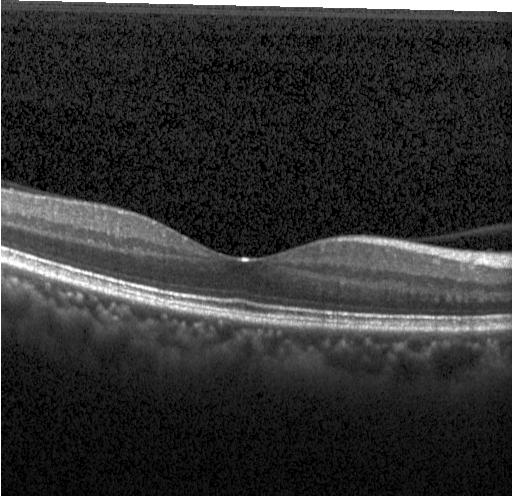

OCT line scan. OCT finding: no choroidal neovascularization, no diabetic macular edema, and no drusen.